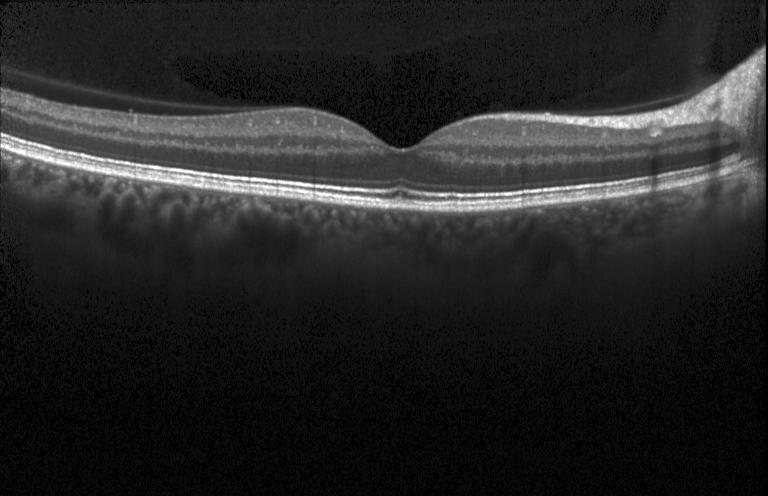 Optical coherence tomography scan.
Finding: no evidence of choroidal neovascularization, diabetic macular edema, or drusen.